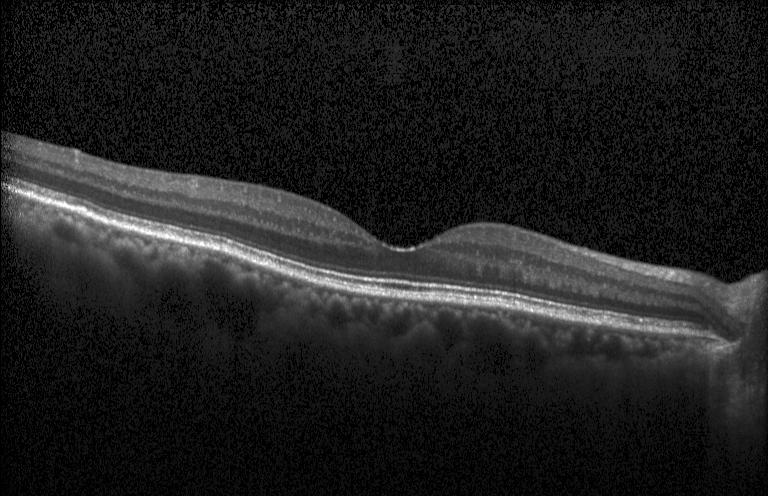 Retinal OCT B-scan, centered on the fovea, Heidelberg Spectralis OCT system, spectral-domain optical coherence tomography. Impression: no evidence of CNV, DME, or drusen.